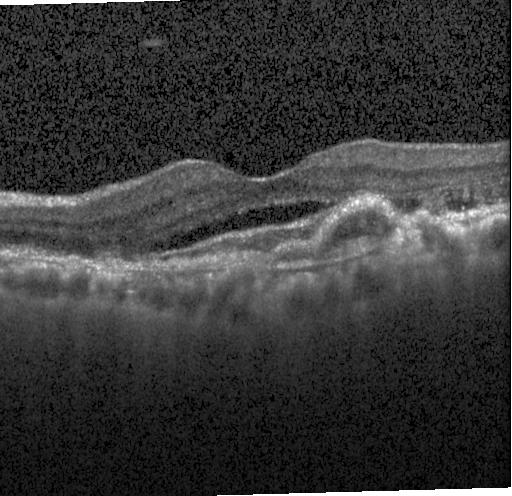 Dx: choroidal neovascularization (CNV).